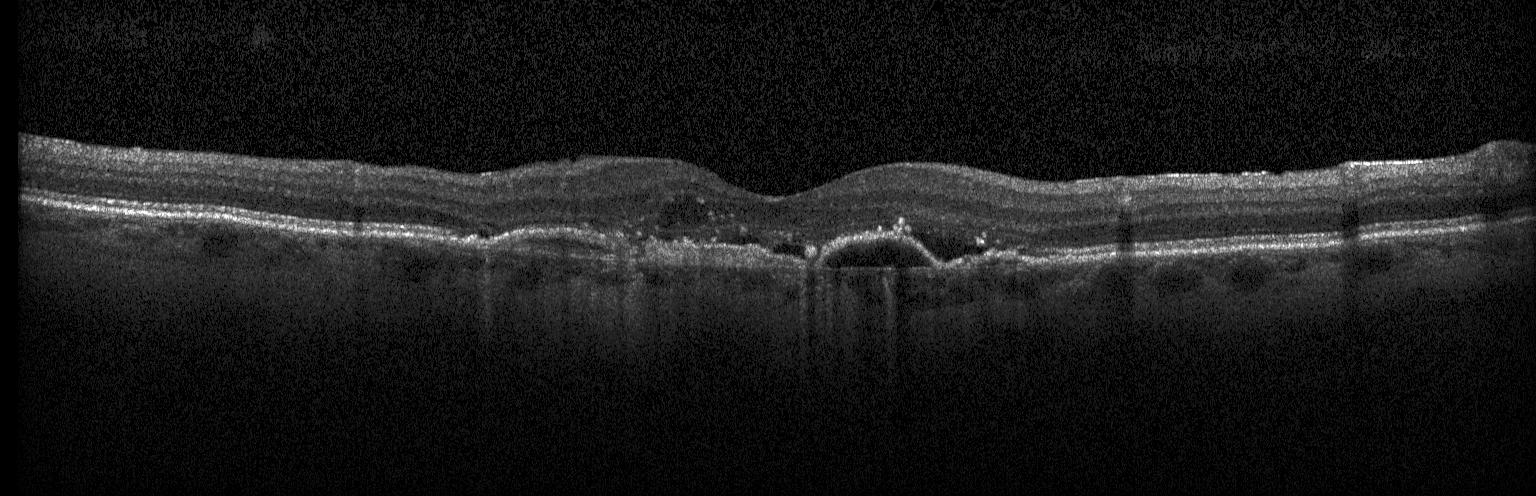

Acquired on a Heidelberg Spectralis. Optical coherence tomography scan.
Macular OCT: a choroidal neovascular membrane.